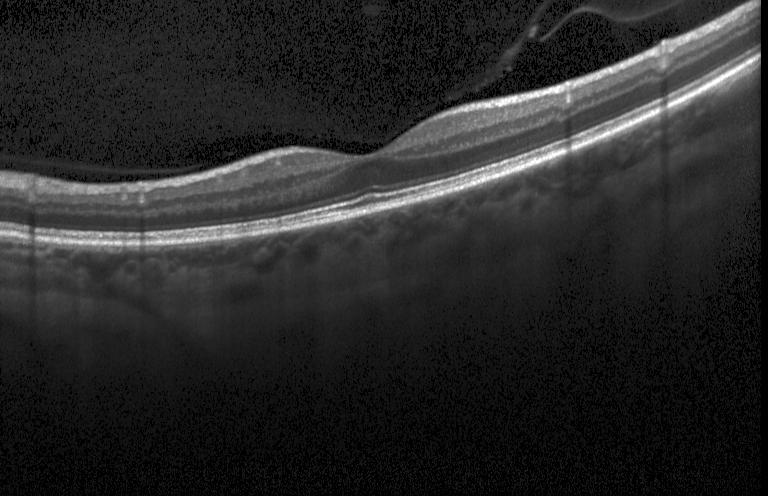

Acquired on a Heidelberg Spectralis, SD-OCT, OCT B-scan.
Finding: no evidence of choroidal neovascularization, diabetic macular edema, or drusen.